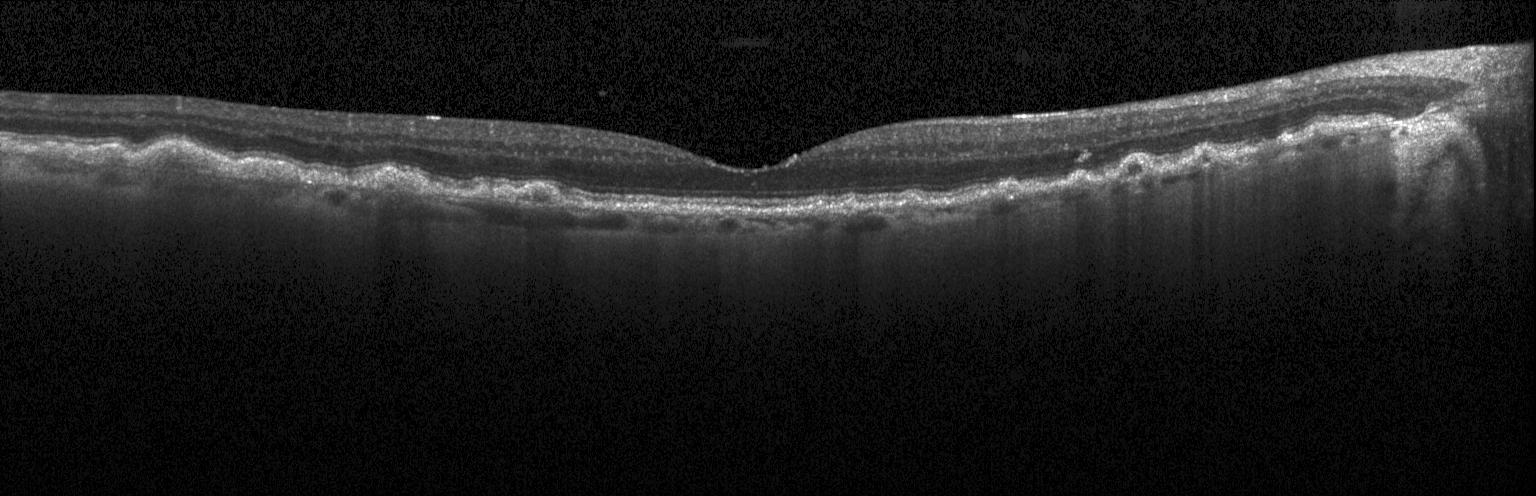
Finding: drusen.